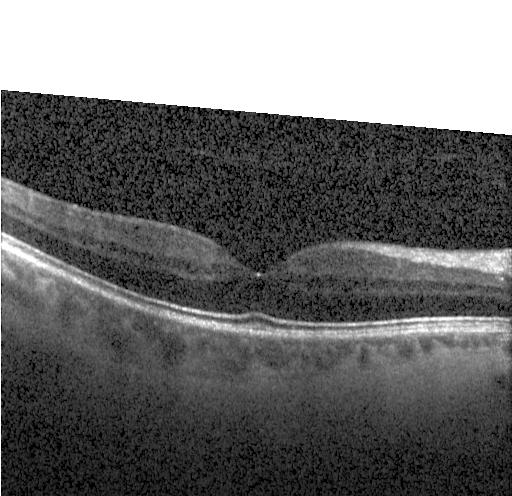
Retinal OCT B-scan · fovea-centered · spectral-domain OCT — The scan shows no choroidal neovascularization, no diabetic macular edema, and no drusen.